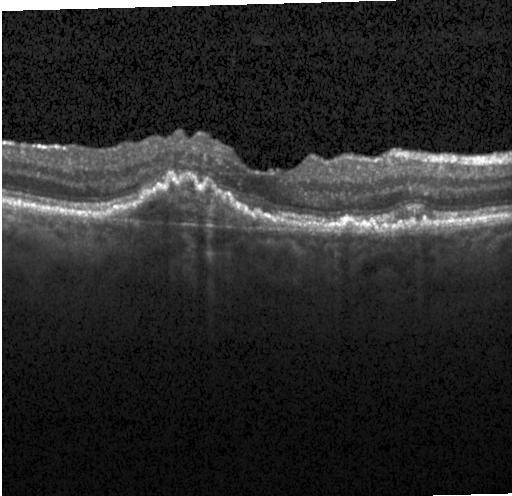 OCT line scan
Assessment: choroidal neovascularization (CNV).